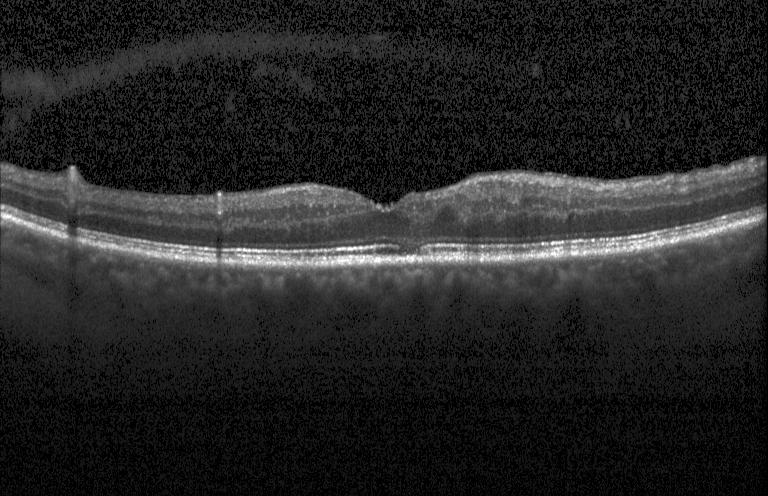
Horizontal scan through the fovea. OCT line scan. SD-OCT — Diagnosis: no choroidal neovascularization, no diabetic macular edema, and no drusen.